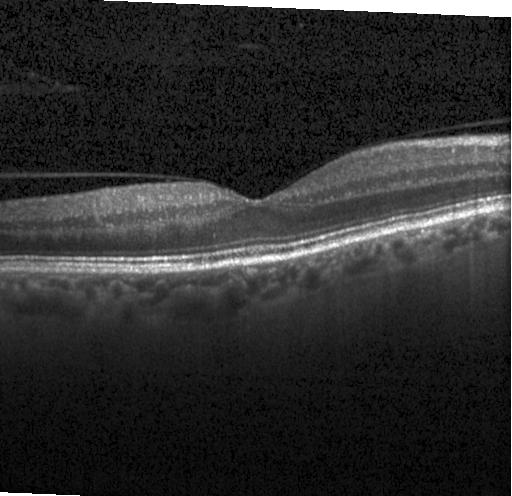 Heidelberg Spectralis. Retinal OCT B-scan. Horizontal scan through the fovea — Impression: no evidence of choroidal neovascularization, diabetic macular edema, or drusen.